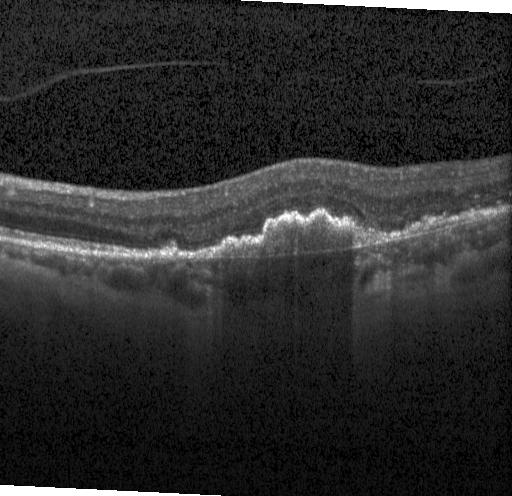

Acquired on a Heidelberg Spectralis. Centered on the fovea. Optical coherence tomography scan. Spectral-domain OCT
Finding: a choroidal neovascular membrane.